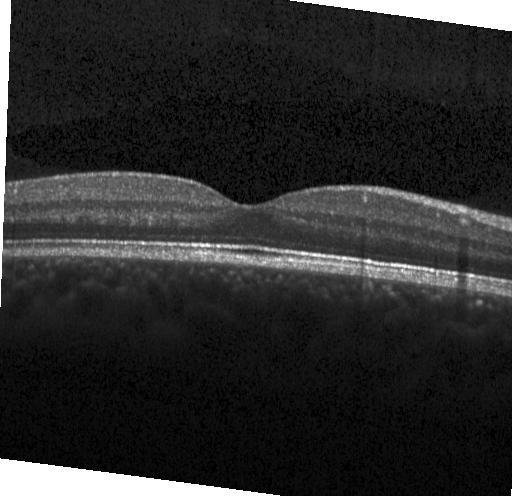 Centered on the fovea · optical coherence tomography scan · instrument: Heidelberg Spectralis — Assessment: no evidence of choroidal neovascularization, diabetic macular edema, or drusen.